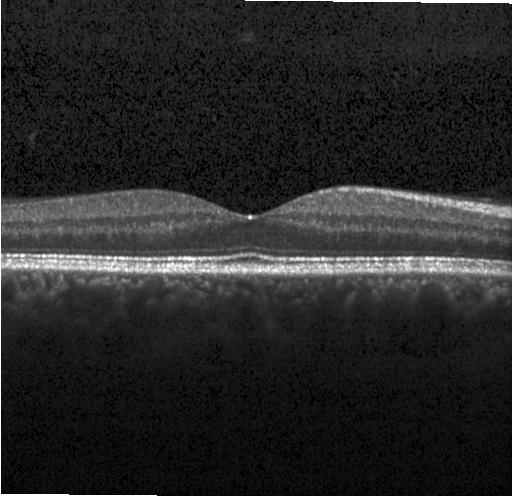
OCT line scan · instrument: Heidelberg Spectralis
Impression: no choroidal neovascularization, diabetic macular edema, or drusen.